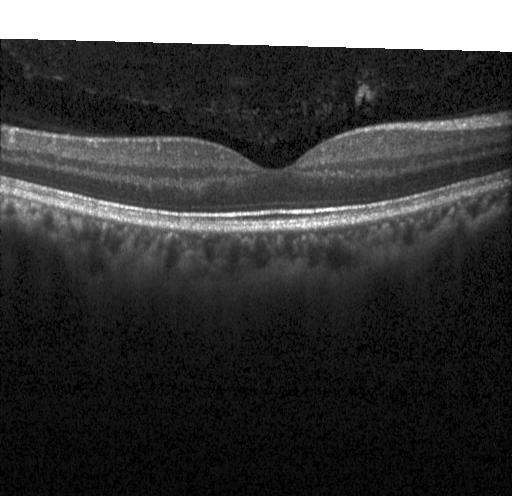 Optical coherence tomography B-scan · Heidelberg Spectralis OCT system · spectral-domain optical coherence tomography. Finding: no choroidal neovascularization, diabetic macular edema, or drusen.